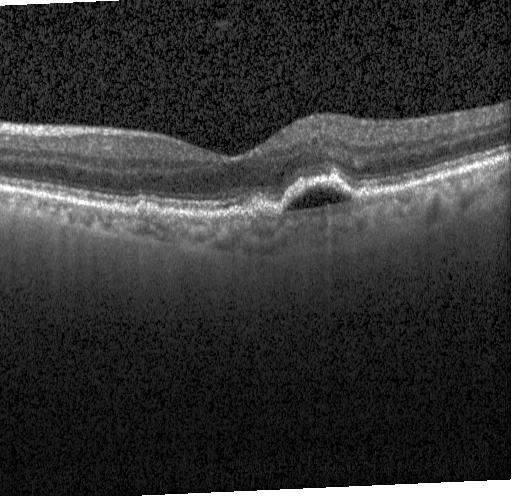

Retinal OCT cross-section showing CNV.